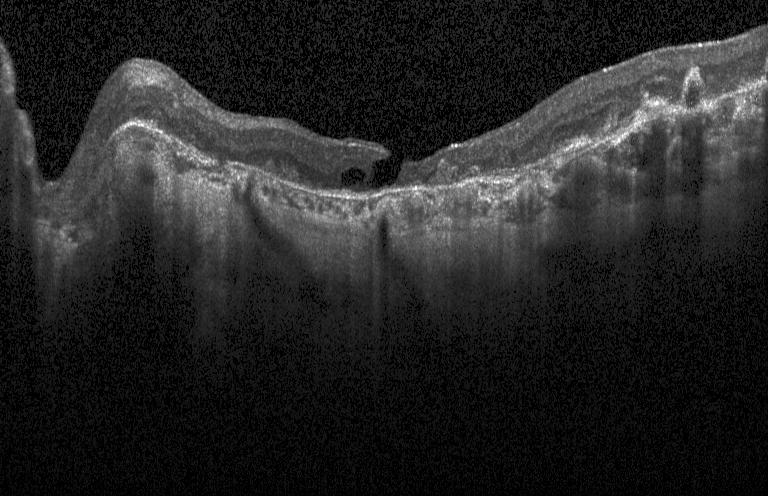 Centered on the fovea; instrument: Heidelberg Spectralis; SD-OCT; optical coherence tomography B-scan — Impression: choroidal neovascularization (CNV).